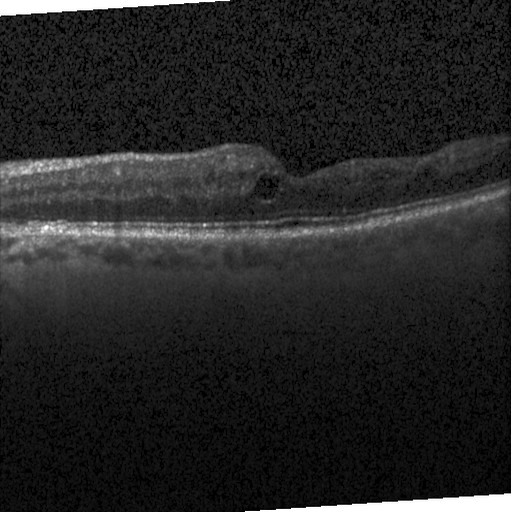 OCT scan showing diabetic macular edema.